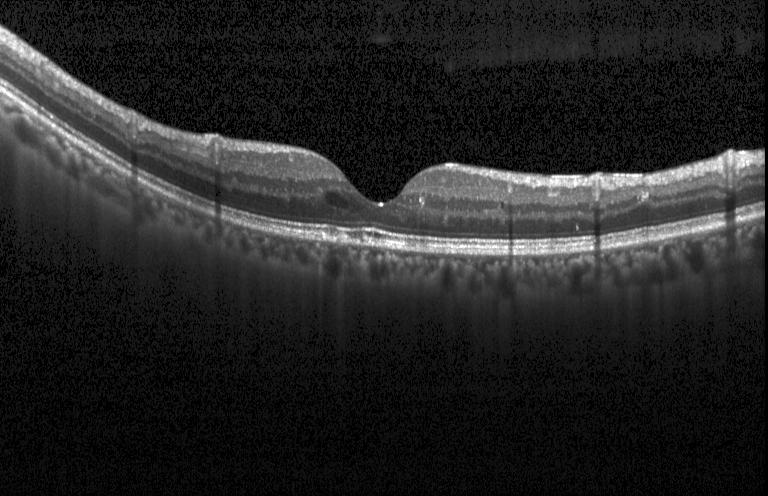

Centered on the fovea, Heidelberg Spectralis OCT system, optical coherence tomography scan, spectral-domain optical coherence tomography.
Dx: diabetic macular edema.